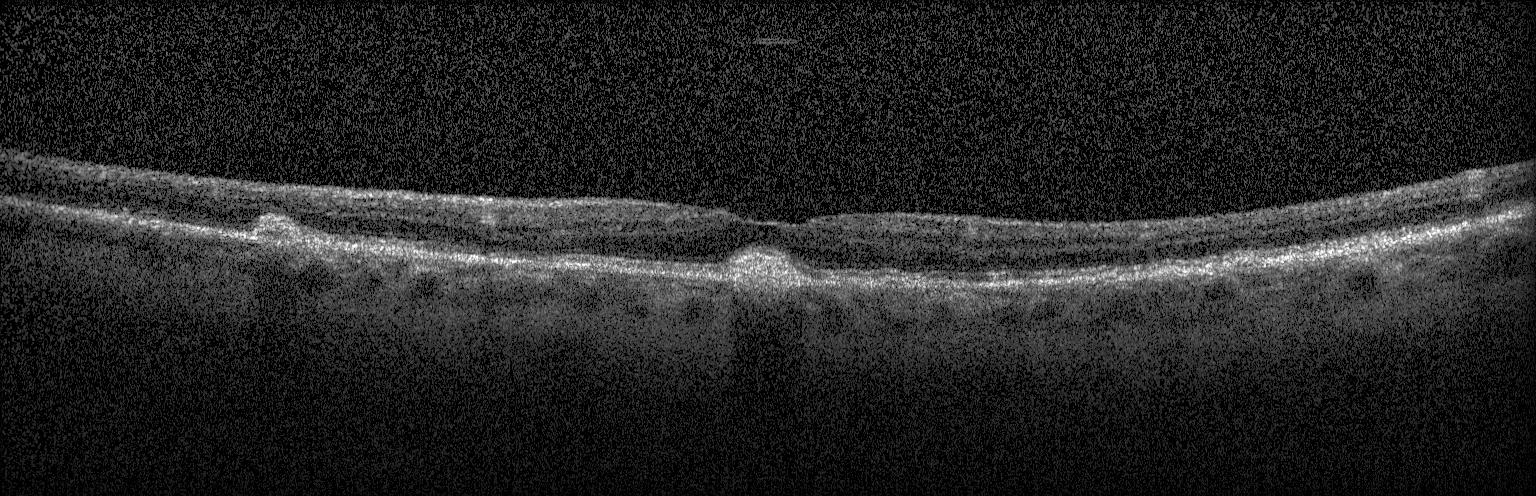

Heidelberg Spectralis OCT system; through the macula; optical coherence tomography B-scan — Impression: multiple drusen.